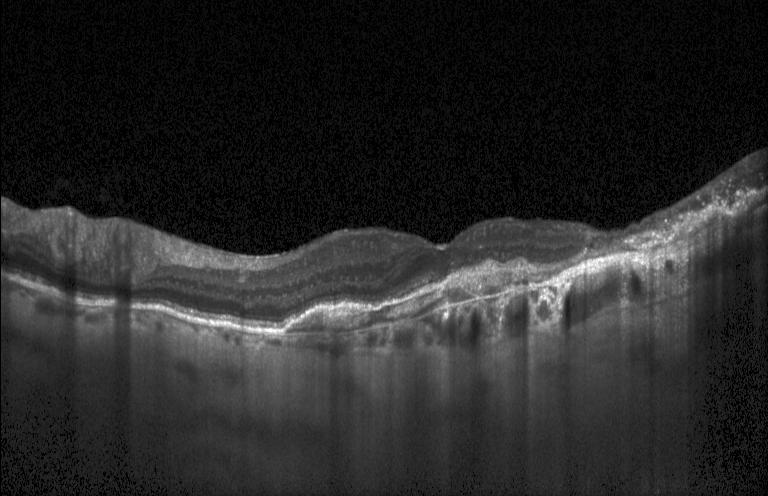
Optical coherence tomography B-scan · spectral-domain OCT — The scan shows choroidal neovascularization.